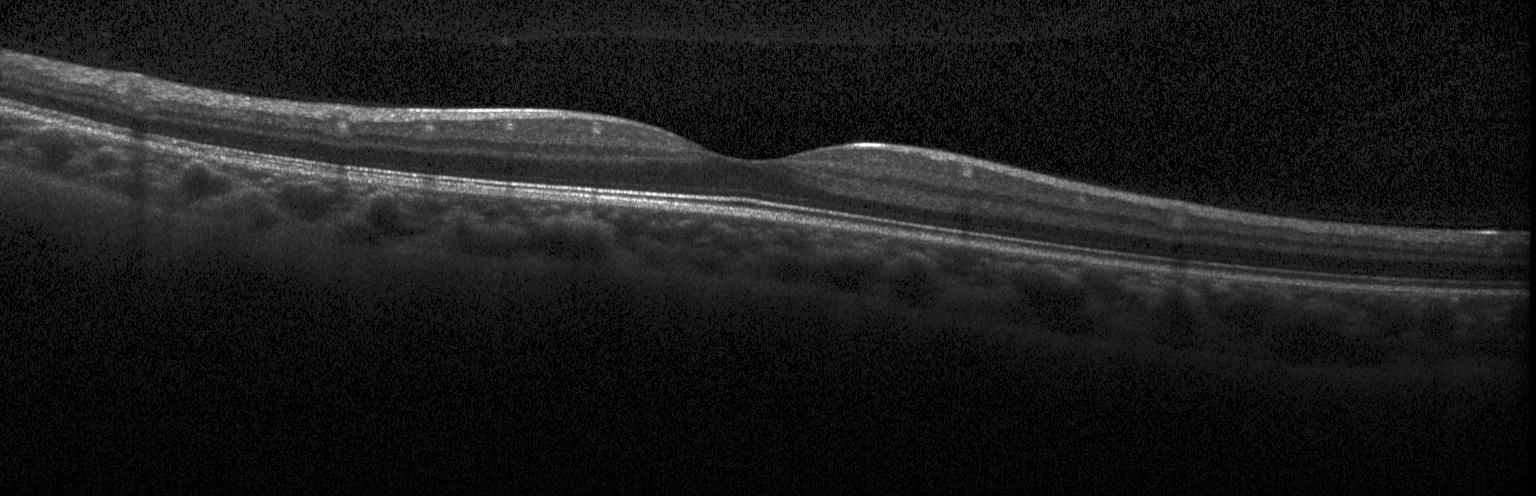

Assessment: neither CNV, DME, nor drusen.